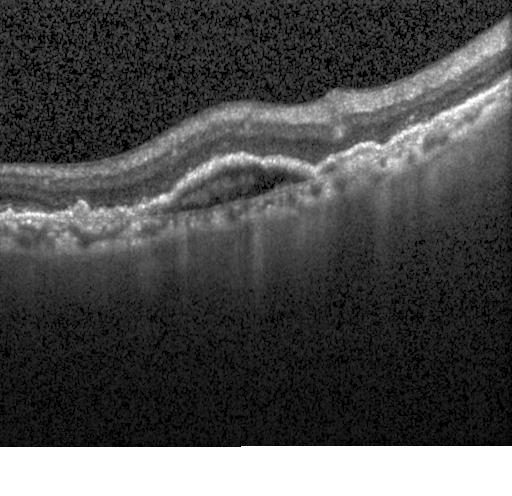

OCT B-scan. Assessment: a choroidal neovascular membrane.